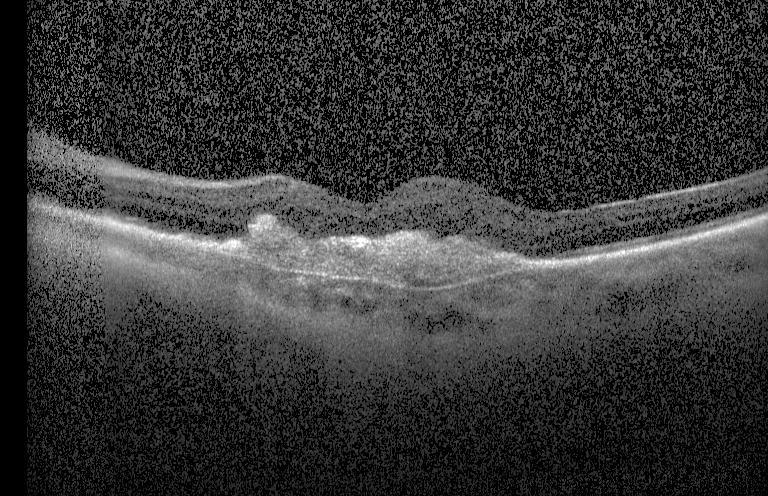
Retinal OCT cross-section showing a choroidal neovascular membrane.